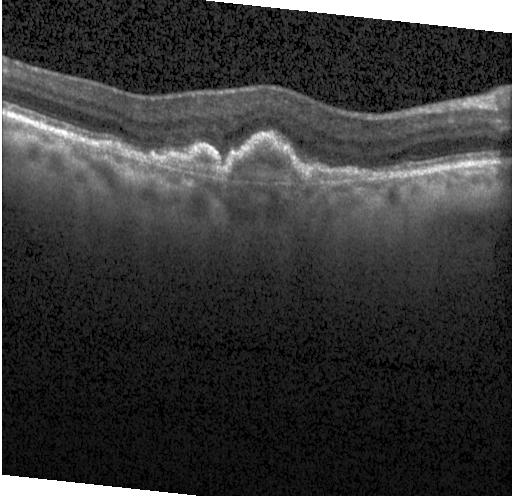 Through the macula, Heidelberg Spectralis OCT system, spectral-domain optical coherence tomography, optical coherence tomography scan.
Finding: CNV.